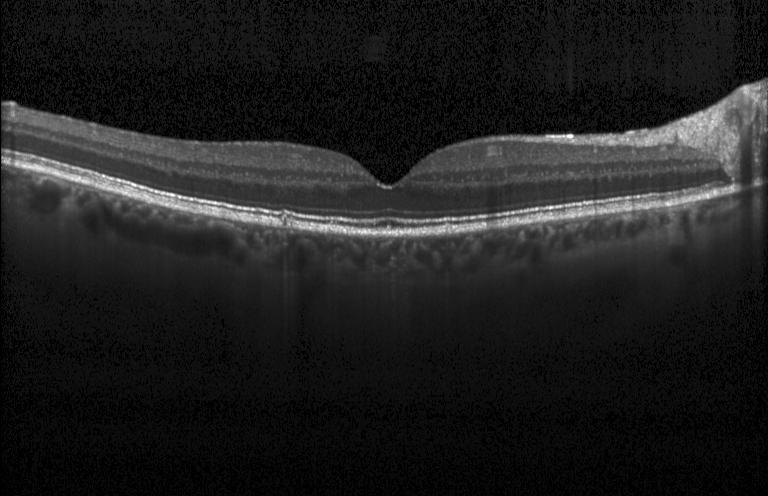

Spectral-domain OCT, fovea-centered, optical coherence tomography B-scan, acquired on a Heidelberg Spectralis.
Diagnosis: no choroidal neovascularization, diabetic macular edema, or drusen.